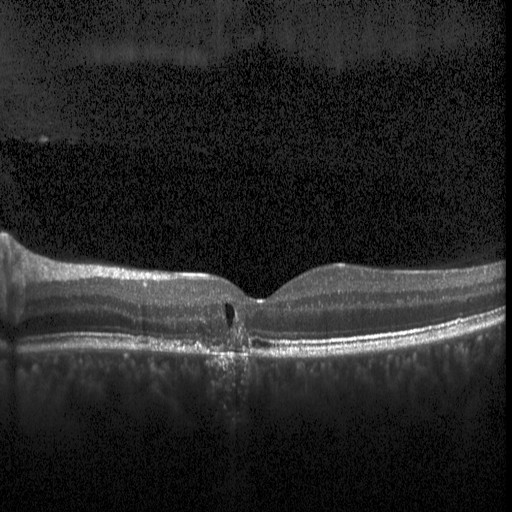
Heidelberg Spectralis OCT system · retinal OCT B-scan.
Assessment: diabetic macular edema (DME).